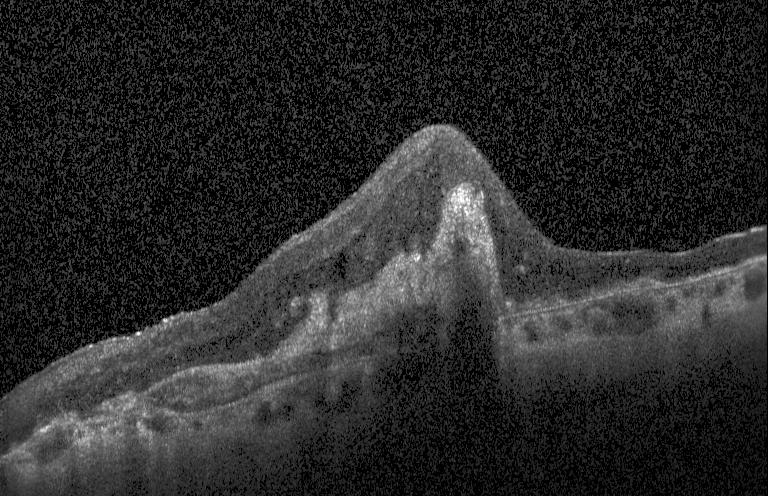 Fovea-centered. OCT line scan
OCT finding: CNV.